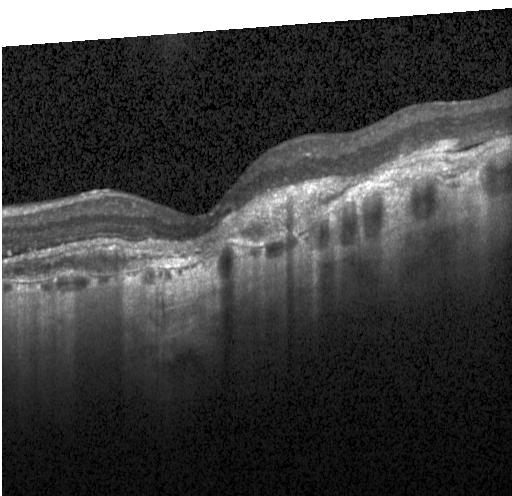

Macular OCT demonstrating a choroidal neovascular membrane.